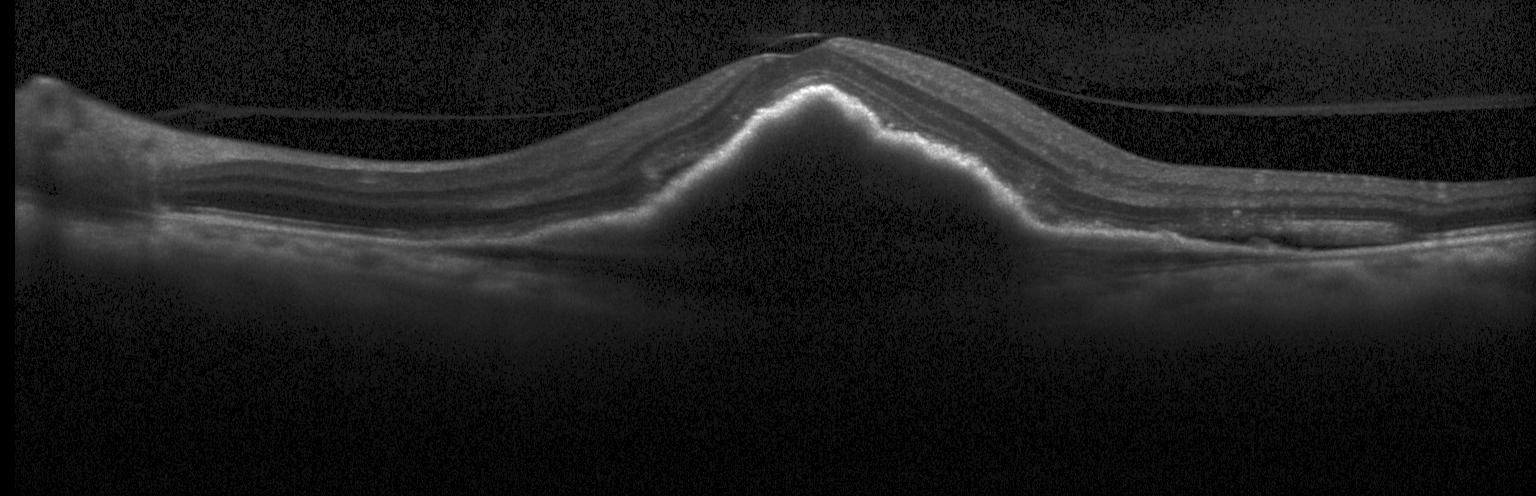
OCT scan showing a choroidal neovascular membrane.